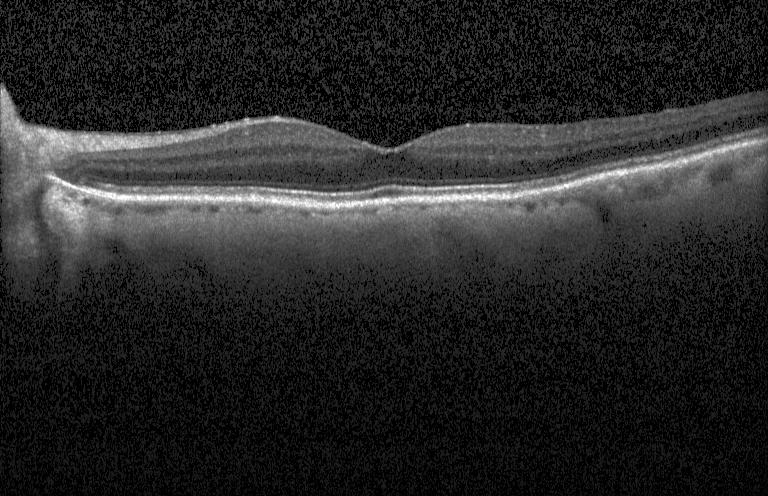 Retinal OCT B-scan — Assessment: neither CNV, DME, nor drusen.